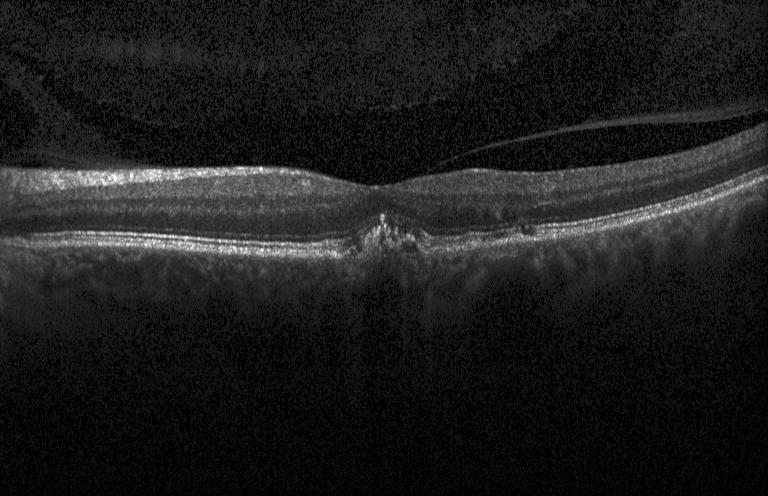 Retinal OCT B-scan · acquired on a Heidelberg Spectralis · through the macula.
The scan shows choroidal neovascularization (CNV).